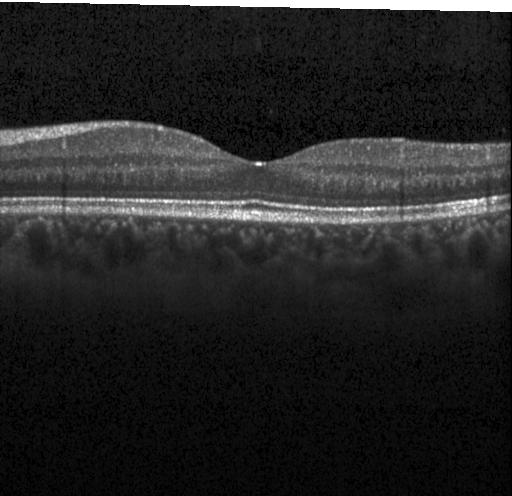
Heidelberg Spectralis, retinal OCT cross-section, spectral-domain OCT.
Finding: no choroidal neovascularization, diabetic macular edema, or drusen.